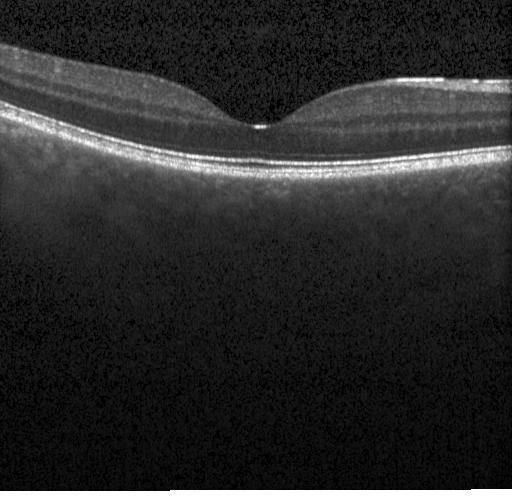

OCT B-scan.
No choroidal neovascularization, diabetic macular edema, or drusen.